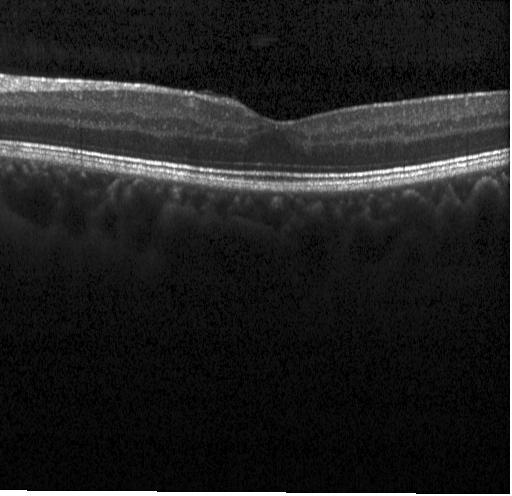 Retinal OCT B-scan — Macular OCT: no choroidal neovascularization, diabetic macular edema, or drusen.